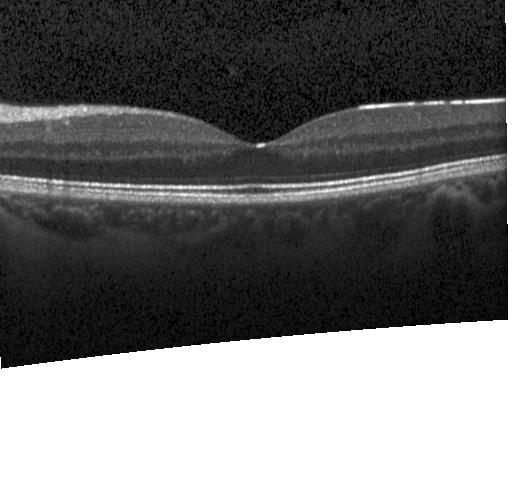

This B-scan demonstrates no choroidal neovascularization, no diabetic macular edema, and no drusen.